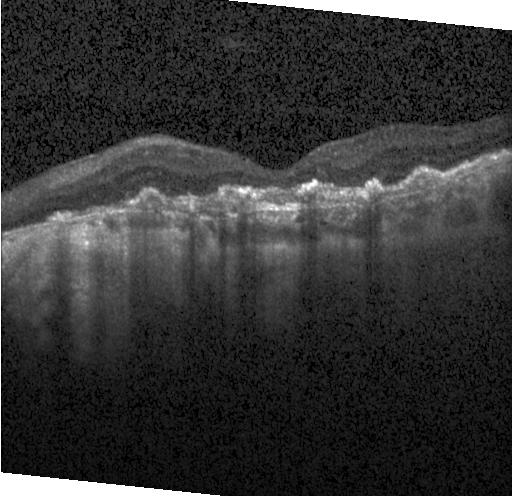
Retinal OCT cross-section showing CNV.